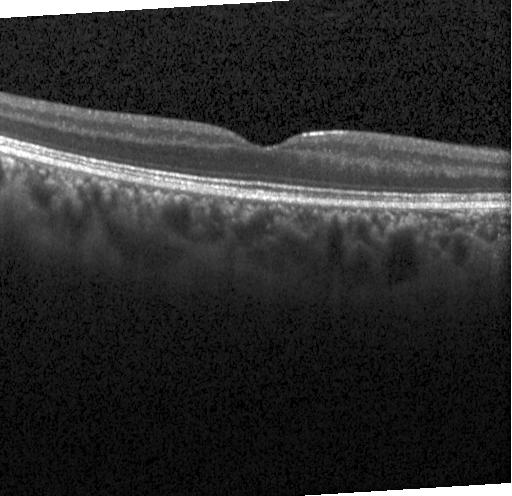
Macular scan · Heidelberg Spectralis OCT system · spectral-domain OCT · optical coherence tomography scan — Dx: neither choroidal neovascularization, diabetic macular edema, nor drusen.